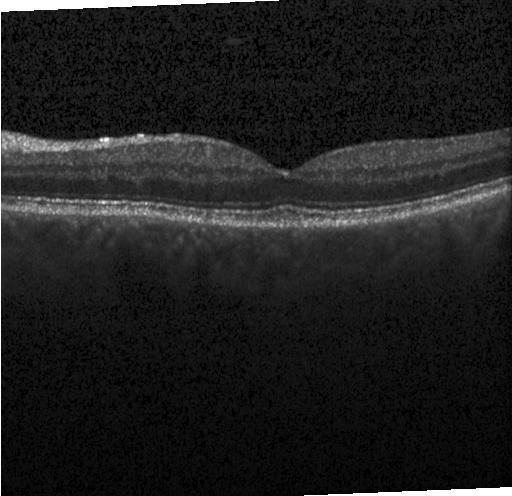
Retinal OCT cross-section; acquired on a Heidelberg Spectralis. No choroidal neovascularization, no diabetic macular edema, and no drusen.